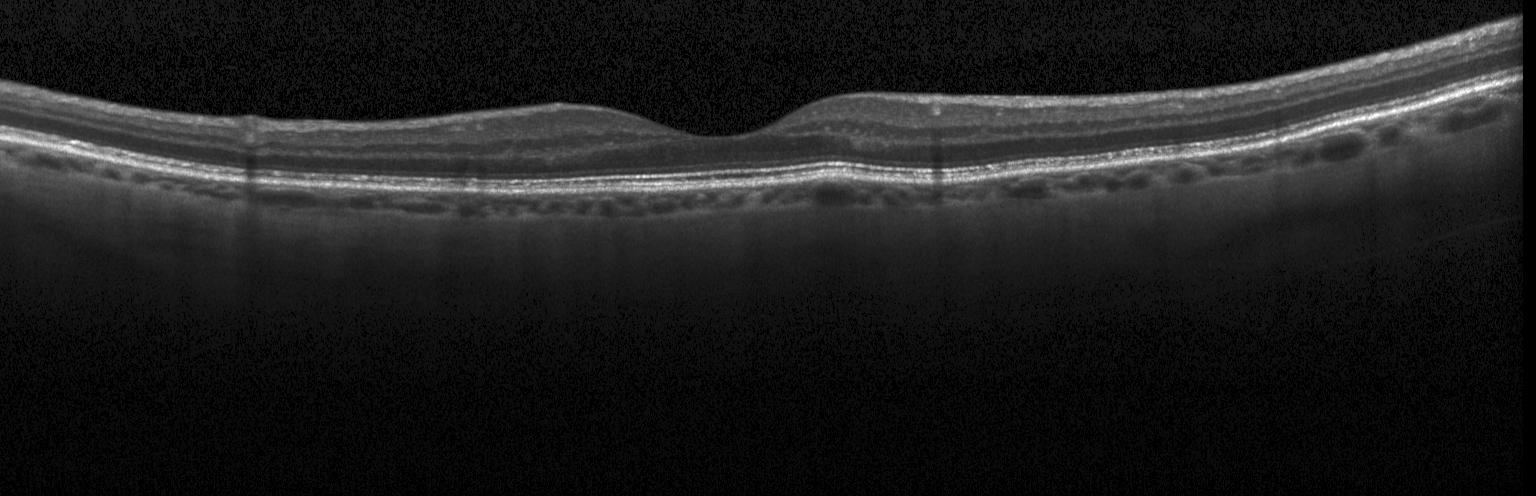
OCT finding: neither choroidal neovascularization, diabetic macular edema, nor drusen.